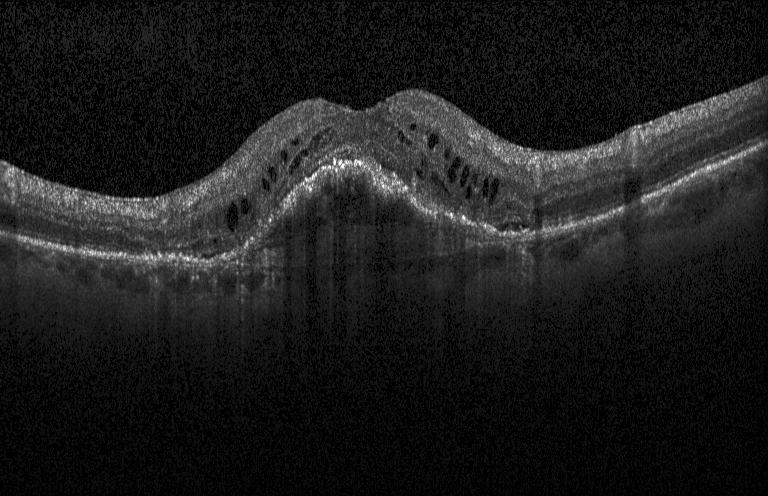

Through the macula; optical coherence tomography B-scan — Diagnosis: a choroidal neovascular membrane.